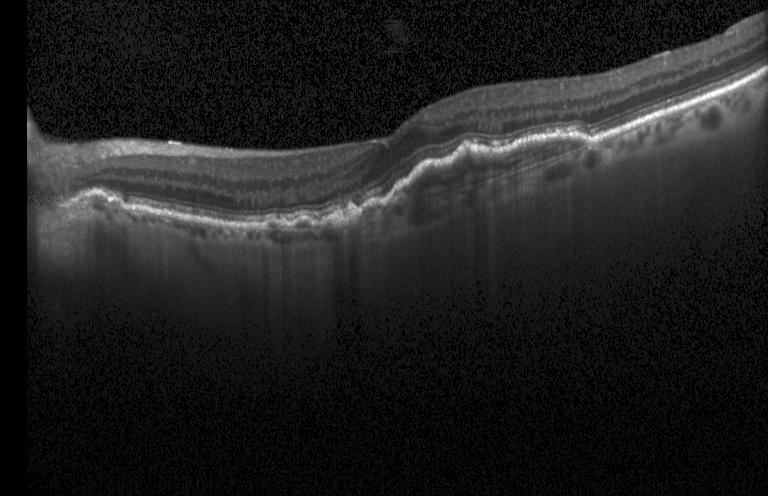

Acquired on a Heidelberg Spectralis. Optical coherence tomography scan — Impression: CNV.